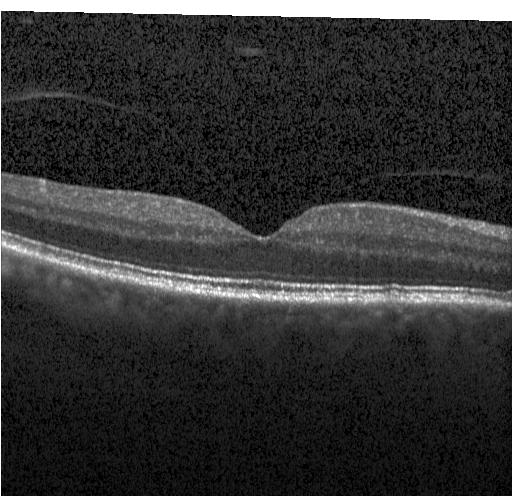 The scan shows no evidence of CNV, DME, or drusen.